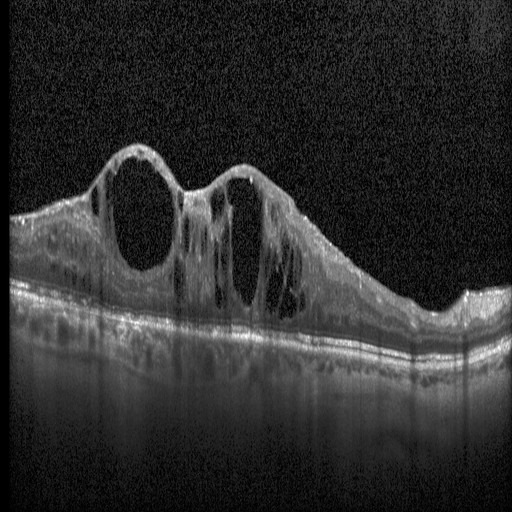 SD-OCT. OCT line scan. Fovea-centered. DME.